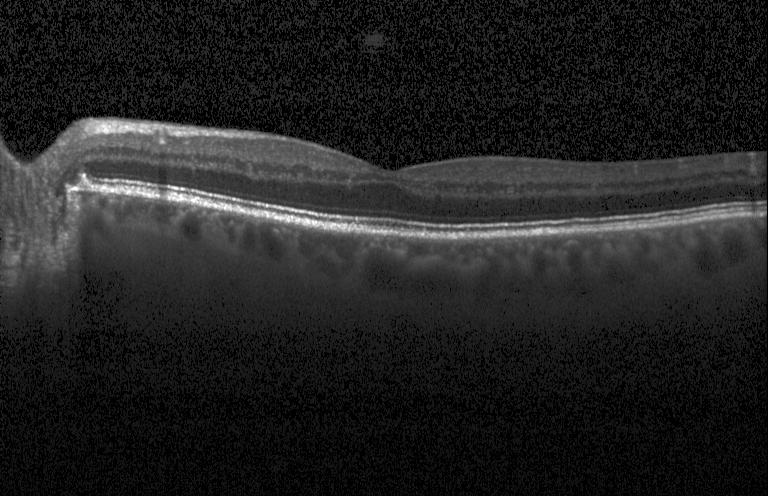 Retinal OCT cross-section showing no evidence of choroidal neovascularization, diabetic macular edema, or drusen.